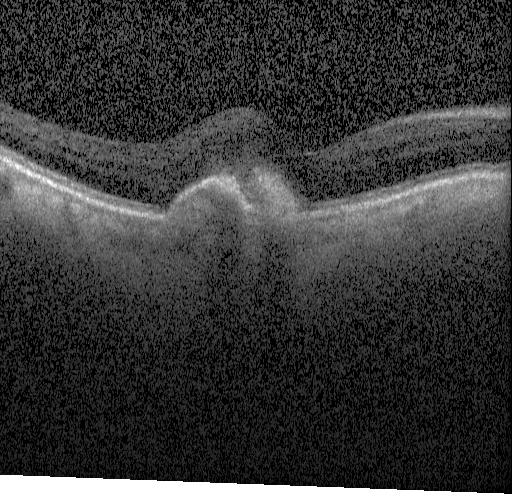

OCT line scan.
Impression: choroidal neovascularization.